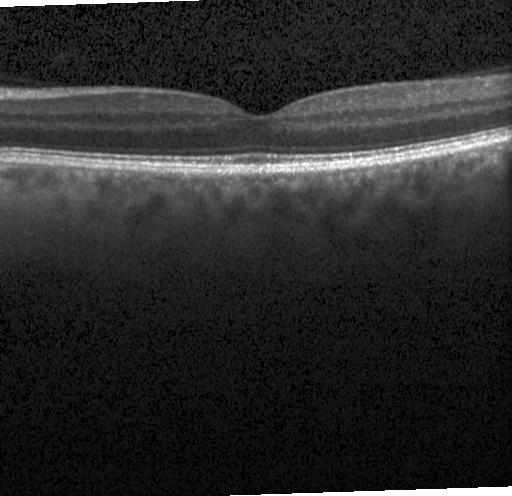 OCT B-scan
Assessment: no choroidal neovascularization, no diabetic macular edema, and no drusen.